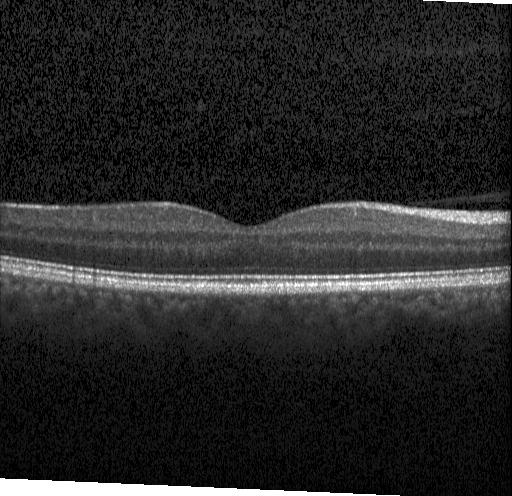 Fovea-centered, OCT B-scan. Diagnosis: neither choroidal neovascularization, diabetic macular edema, nor drusen.